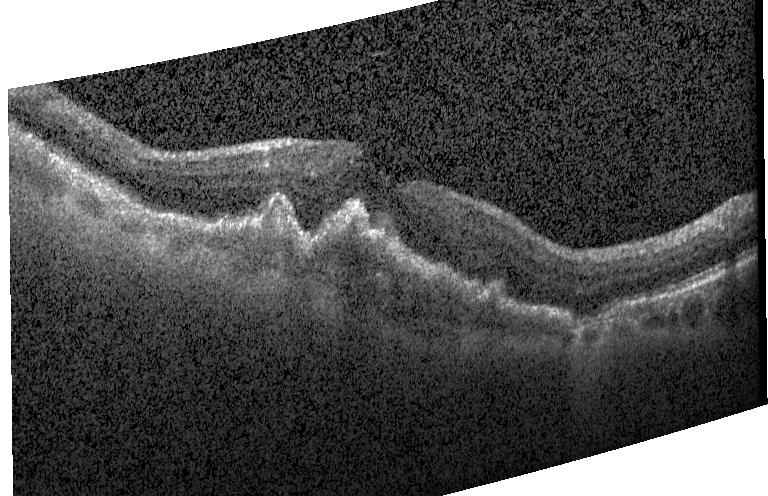

Spectral-domain OCT; instrument: Heidelberg Spectralis; OCT B-scan — Impression: a choroidal neovascular membrane.